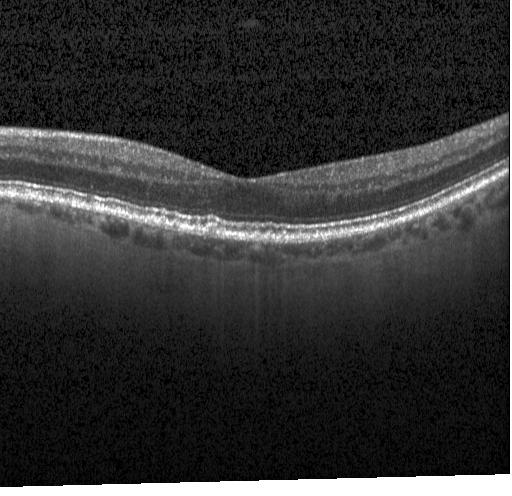
Spectral-domain OCT. Retinal OCT B-scan
Dx: sub-RPE drusenoid deposits.